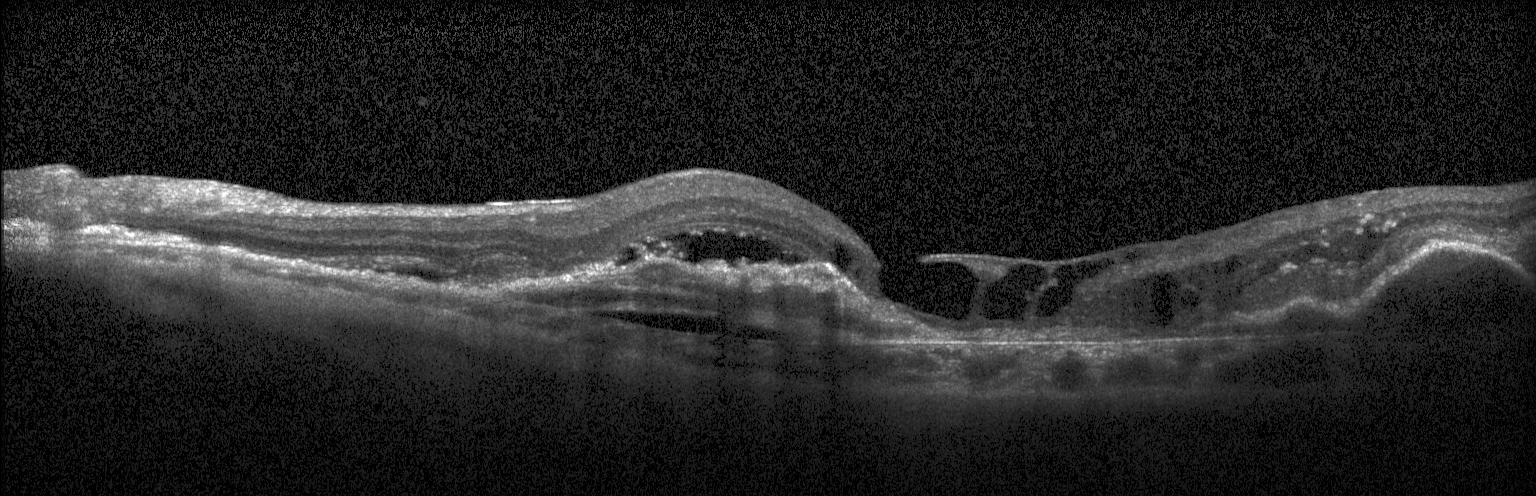
Optical coherence tomography B-scan. Acquired on a Heidelberg Spectralis. Fovea-centered. Spectral-domain optical coherence tomography. Diagnosis: choroidal neovascularization (CNV).